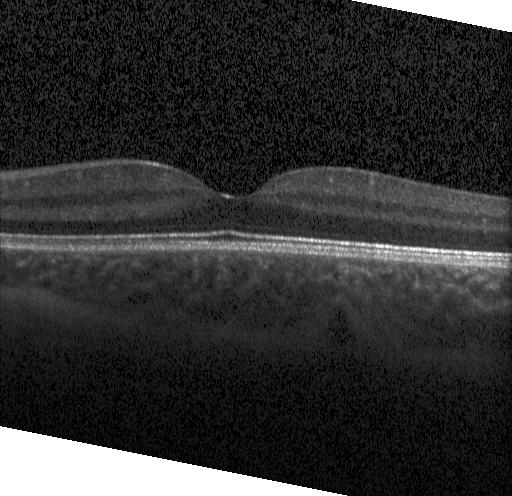 Spectral-domain OCT. Optical coherence tomography B-scan. Heidelberg Spectralis OCT system. Diagnosis: no choroidal neovascularization, no diabetic macular edema, and no drusen.